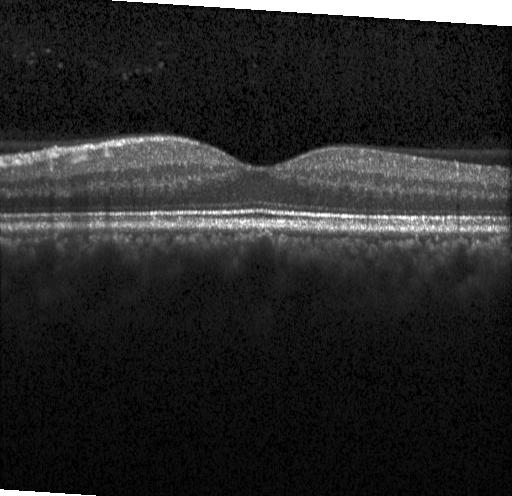 Dx: neither CNV, DME, nor drusen.